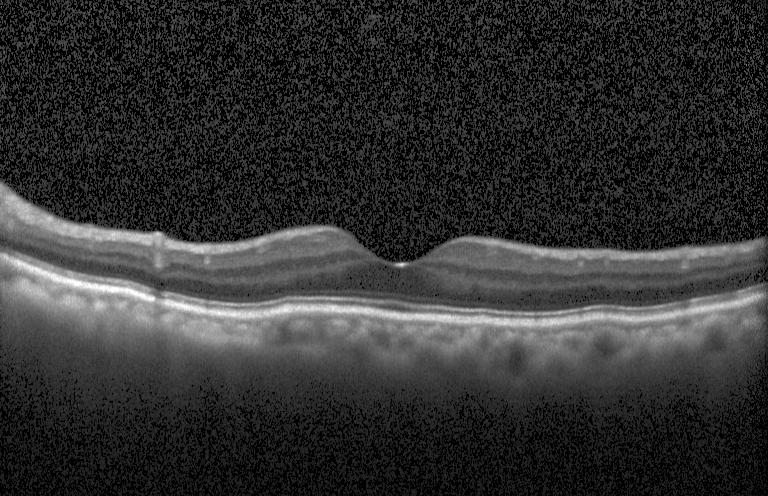

Optical coherence tomography B-scan.
Diagnosis: neither choroidal neovascularization, diabetic macular edema, nor drusen.